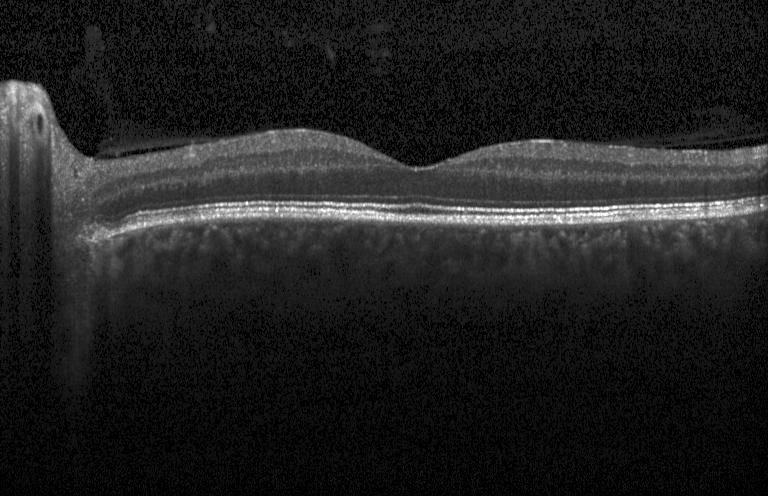
Instrument: Heidelberg Spectralis. Through the macula. Spectral-domain OCT. Optical coherence tomography scan
Macular OCT: no CNV, DME, or drusen.